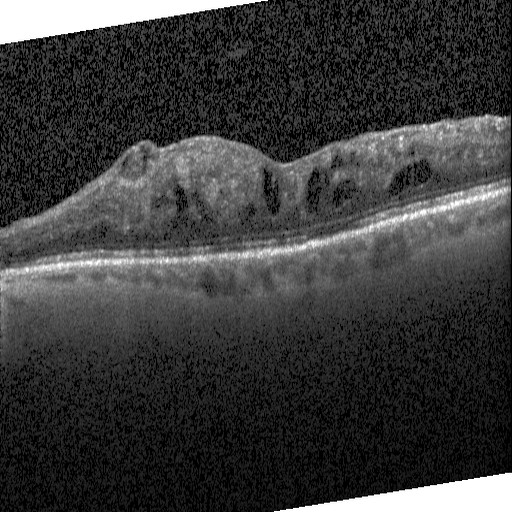 Through the macula · optical coherence tomography B-scan · Heidelberg Spectralis · spectral-domain OCT.
Diabetic macular edema.